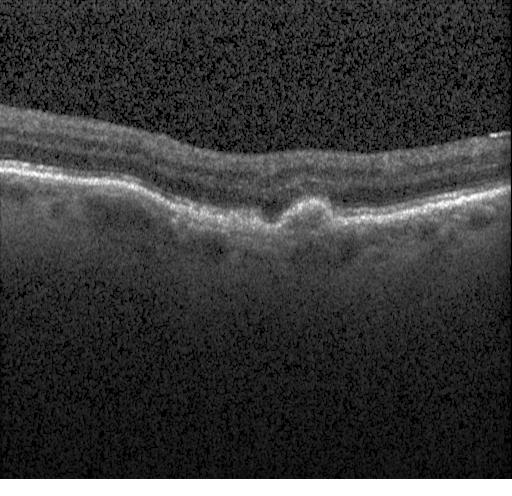
Heidelberg Spectralis OCT system, optical coherence tomography scan.
OCT finding: CNV.